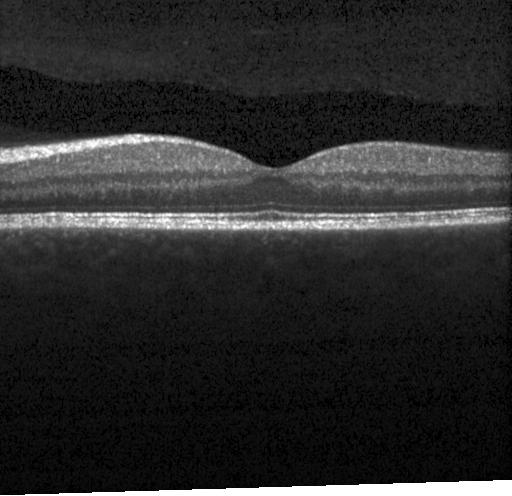
Heidelberg Spectralis OCT system, retinal OCT cross-section. Impression: no choroidal neovascularization, no diabetic macular edema, and no drusen.